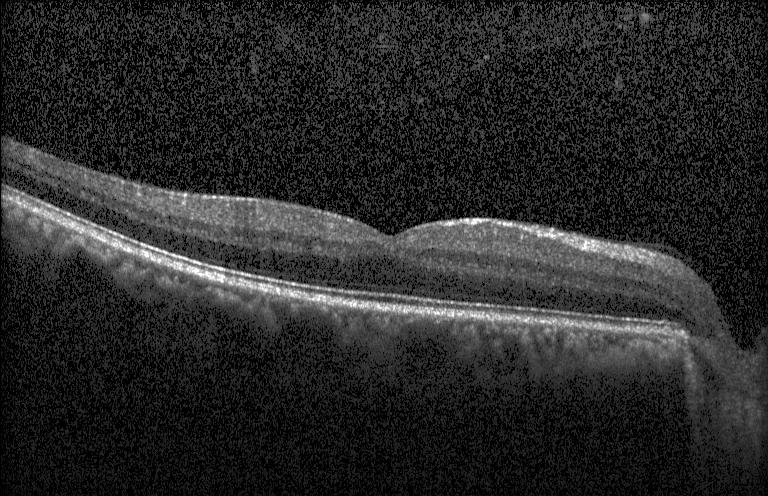

Retinal OCT cross-section showing no evidence of choroidal neovascularization, diabetic macular edema, or drusen.